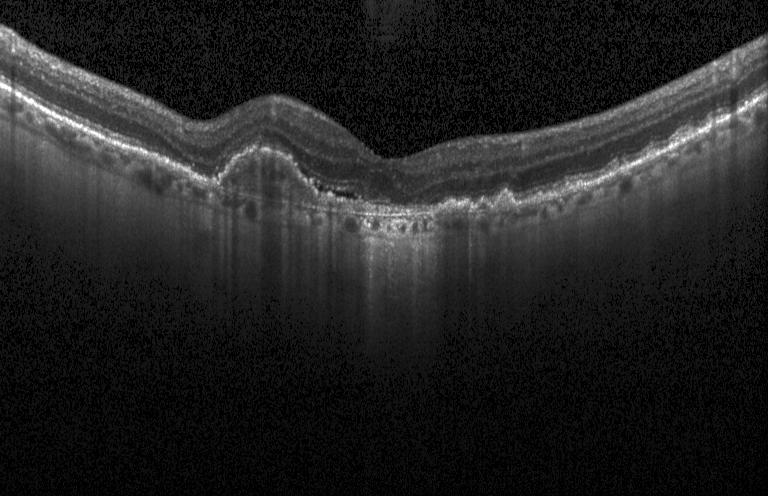

OCT B-scan. Macular scan. Spectral-domain optical coherence tomography.
Finding: choroidal neovascularization (CNV).